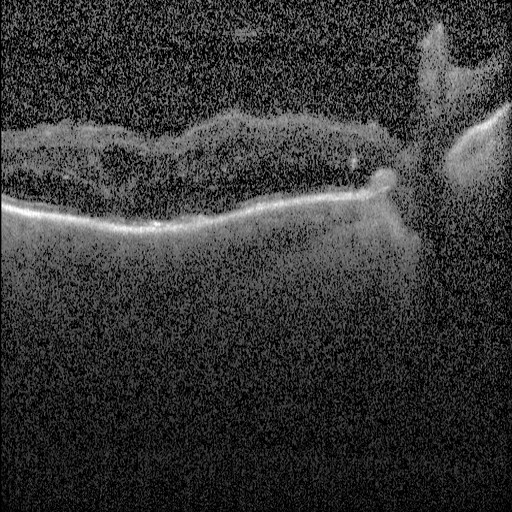
Spectral-domain OCT B-scan: diabetic macular edema.